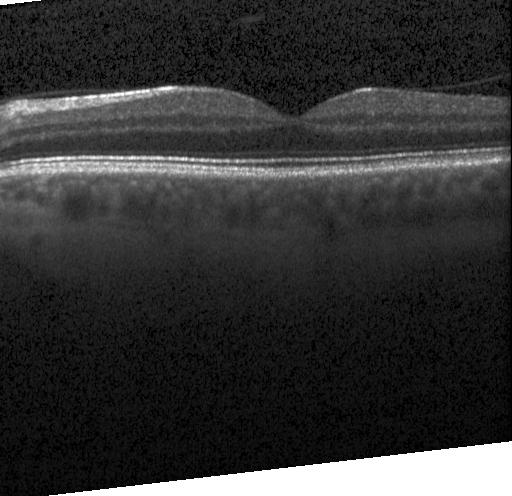 OCT line scan, Heidelberg Spectralis OCT system — Macular OCT: no choroidal neovascularization, diabetic macular edema, or drusen.